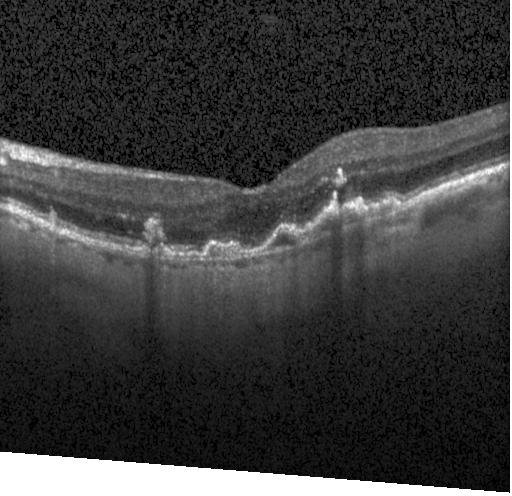
OCT finding: choroidal neovascularization.